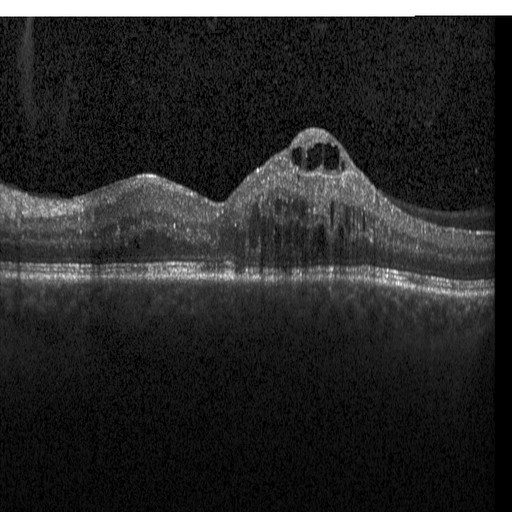
Retinal OCT cross-section; through the macula; spectral-domain OCT; acquired on a Heidelberg Spectralis — The scan shows diabetic macular edema.